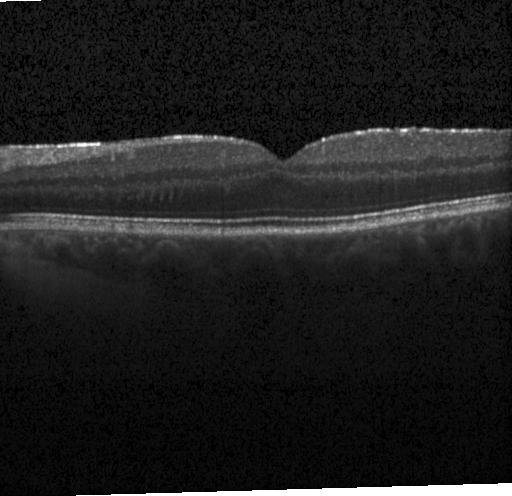

Optical coherence tomography B-scan; spectral-domain OCT; acquired on a Heidelberg Spectralis; horizontal scan through the fovea — Impression: no evidence of choroidal neovascularization, diabetic macular edema, or drusen.